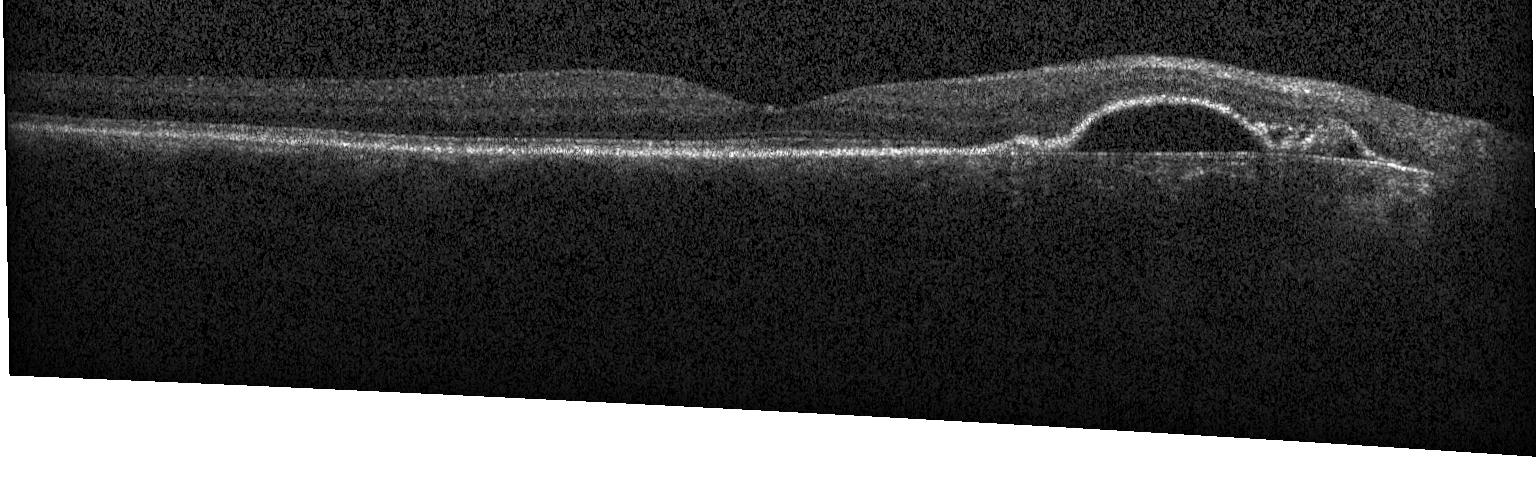 Macular OCT: a choroidal neovascular membrane.